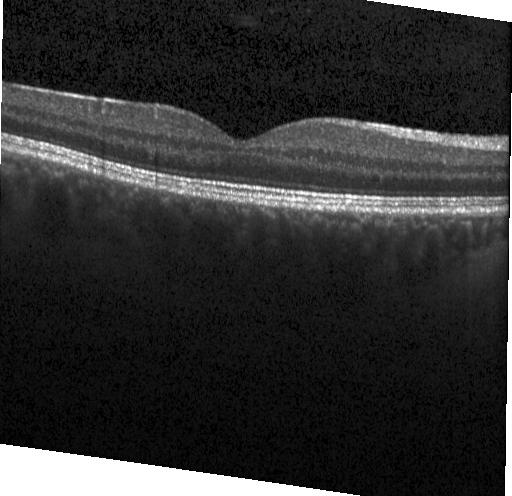 Optical coherence tomography scan
Assessment: no CNV, no DME, and no drusen.